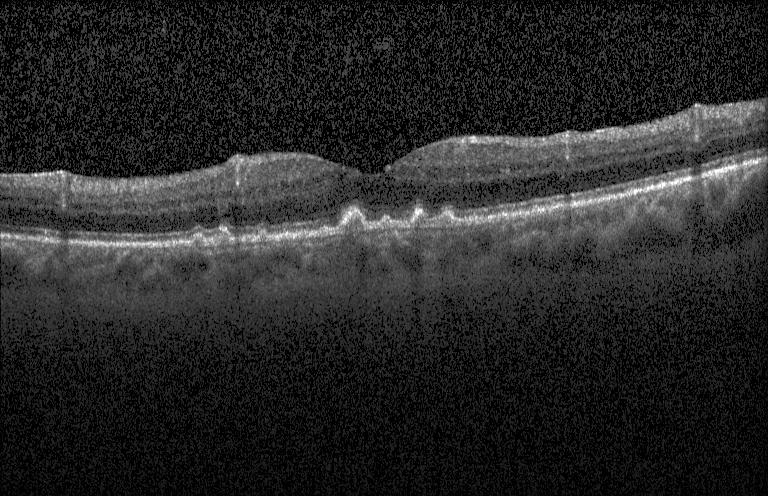
Impression: drusen.